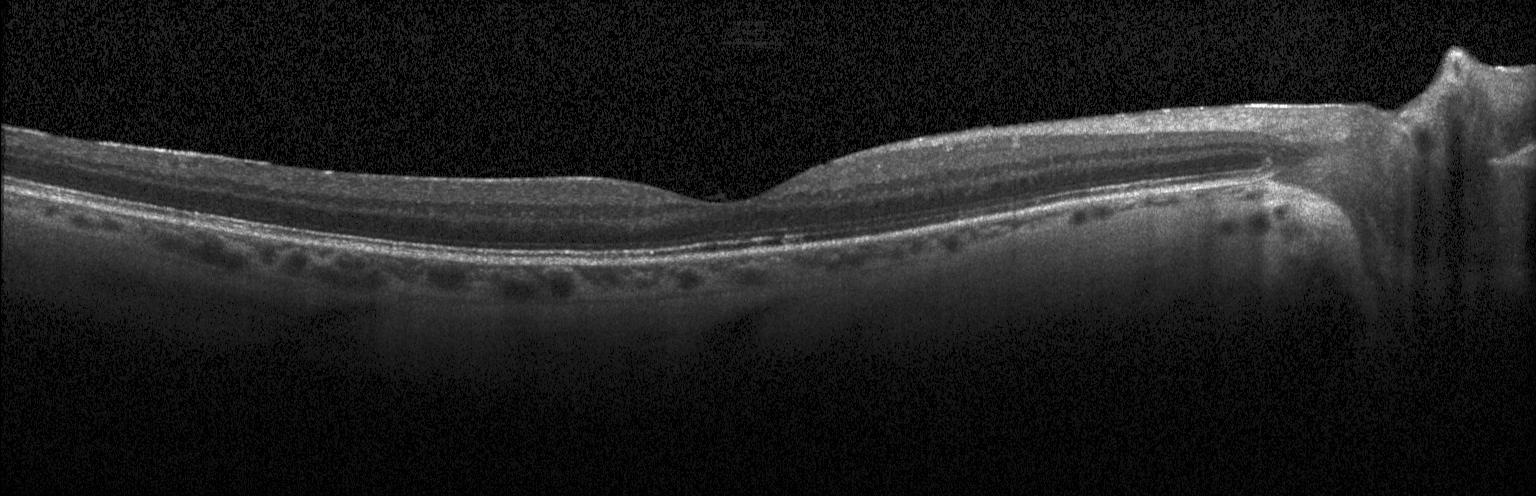

Optical coherence tomography B-scan — The scan shows neither choroidal neovascularization, diabetic macular edema, nor drusen.